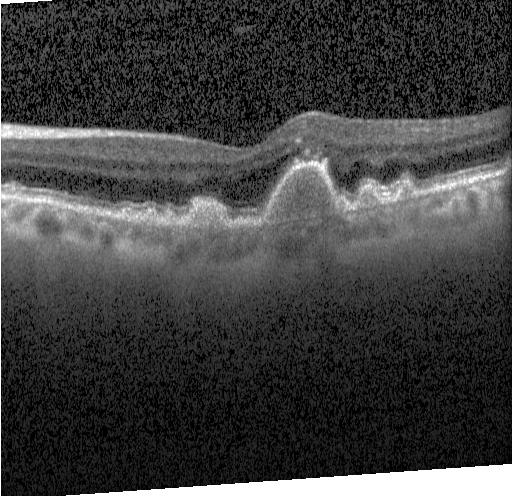

Centered on the fovea · Heidelberg Spectralis · retinal OCT cross-section · SD-OCT.
OCT finding: multiple drusen.